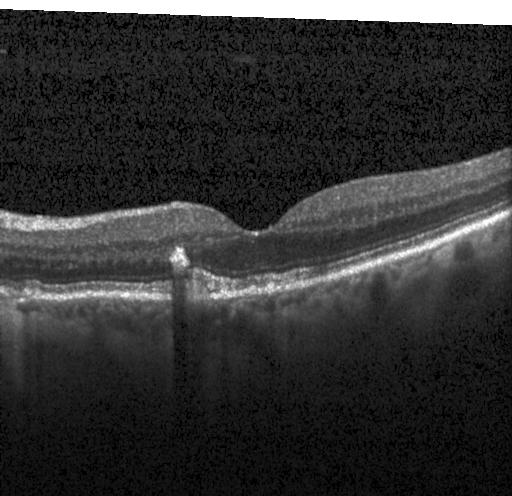 Acquired on a Heidelberg Spectralis · through the macula · spectral-domain OCT · retinal OCT cross-section.
Finding: sub-RPE drusenoid deposits.